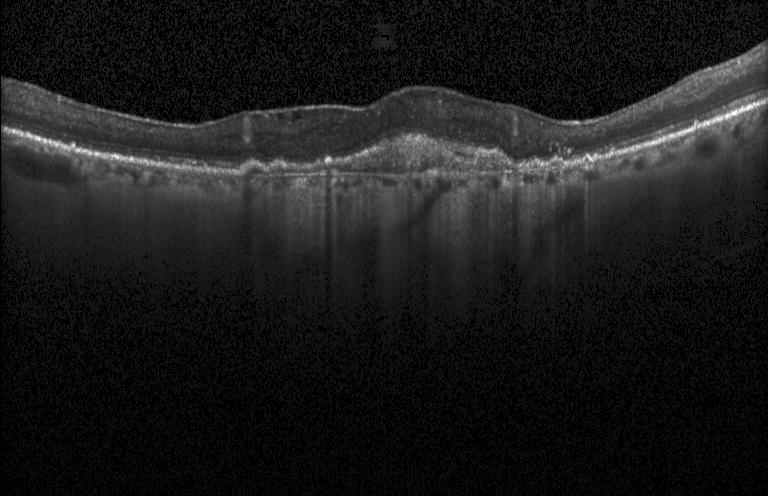 Acquired on a Heidelberg Spectralis, spectral-domain OCT, OCT line scan, macular scan
Macular OCT: choroidal neovascularization (CNV).